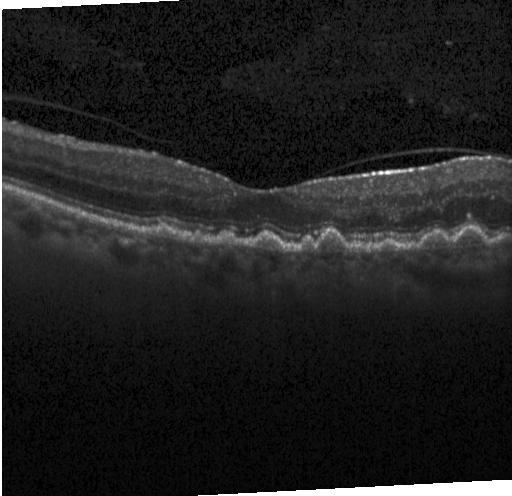

This B-scan demonstrates choroidal neovascularization.